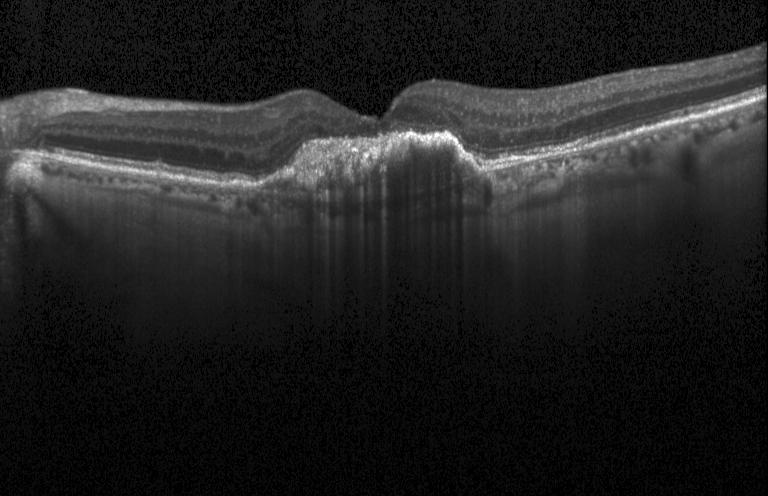

Spectral-domain optical coherence tomography, OCT line scan, through the macula. Macular OCT: a choroidal neovascular membrane.